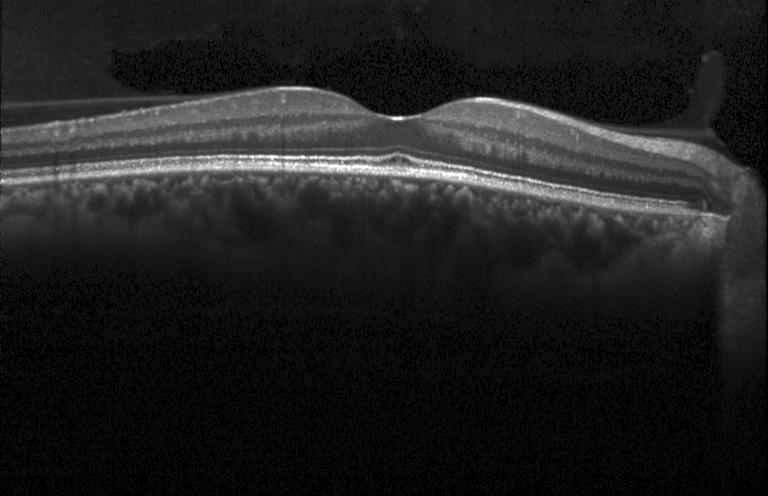
Macular OCT: no choroidal neovascularization, no diabetic macular edema, and no drusen.